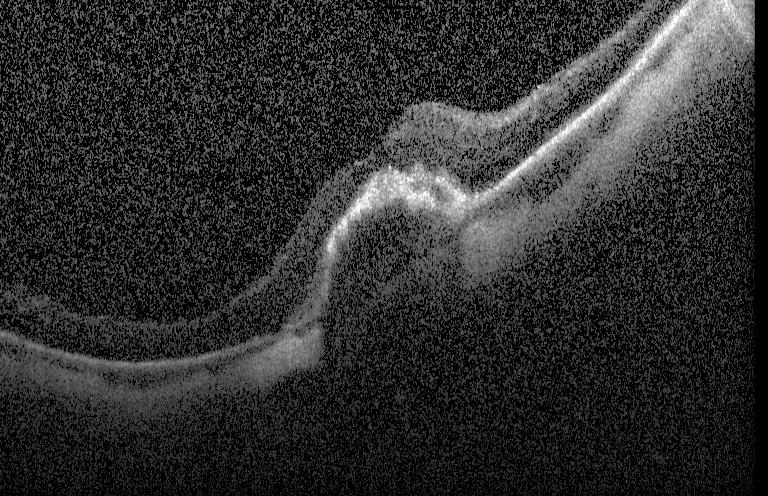

Spectral-domain optical coherence tomography; OCT B-scan. Impression: a choroidal neovascular membrane.